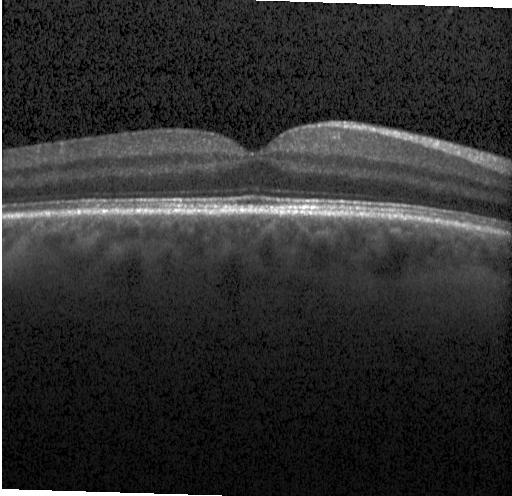

Retinal OCT B-scan. Assessment: no choroidal neovascularization, no diabetic macular edema, and no drusen.